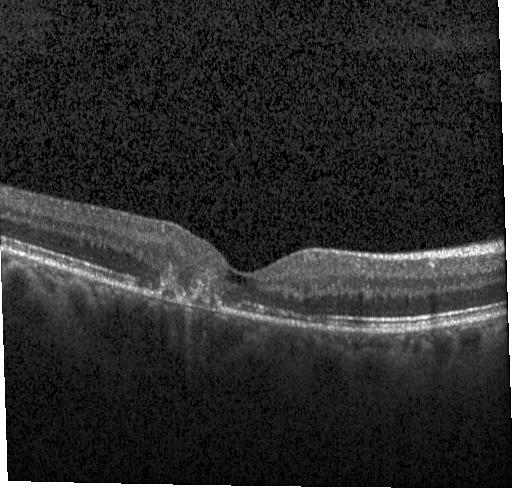
OCT B-scan · spectral-domain OCT · macular scan
Dx: CNV.